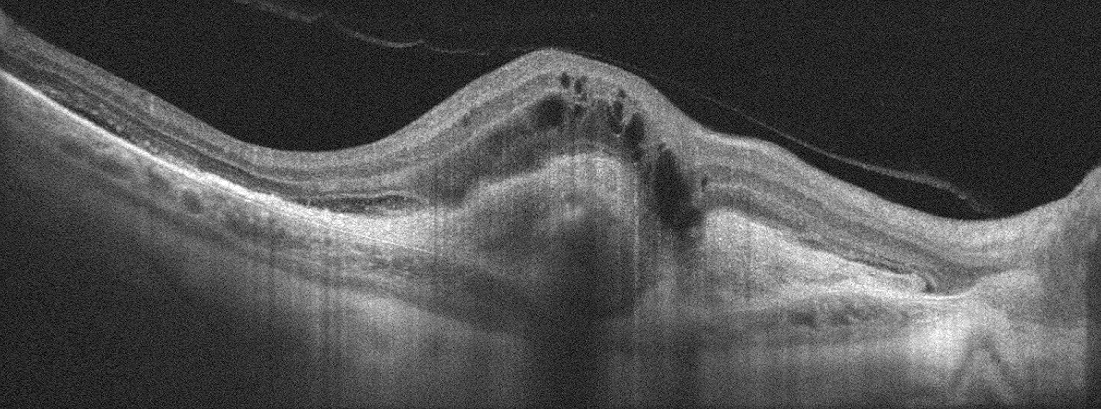

Macular scan · acquired on an Optovue Avanti RTVue XR · OCT line scan — OCT finding: age-related macular degeneration.